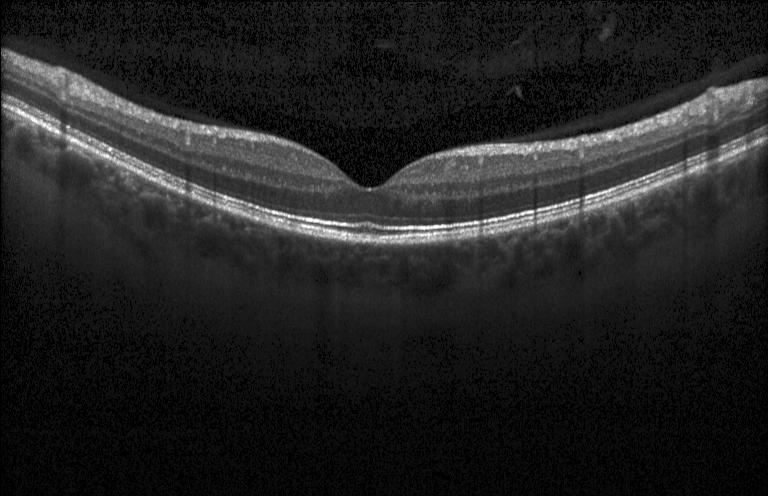
Optical coherence tomography scan
This B-scan demonstrates no choroidal neovascularization, no diabetic macular edema, and no drusen.